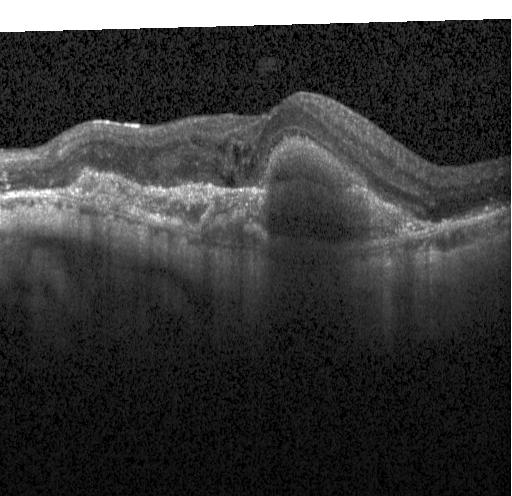
OCT line scan · horizontal scan through the fovea · Heidelberg Spectralis OCT system. Finding: a choroidal neovascular membrane.